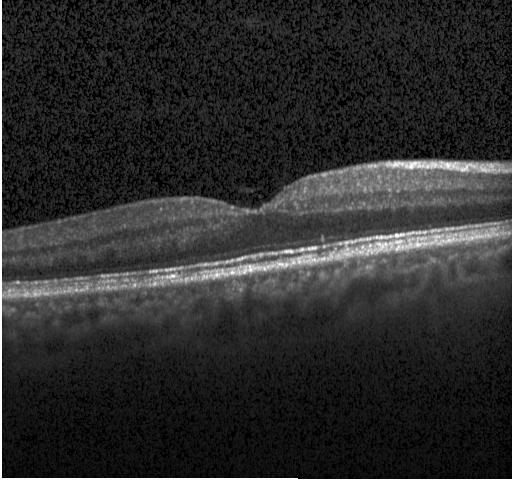 Diagnosis: no evidence of CNV, DME, or drusen.